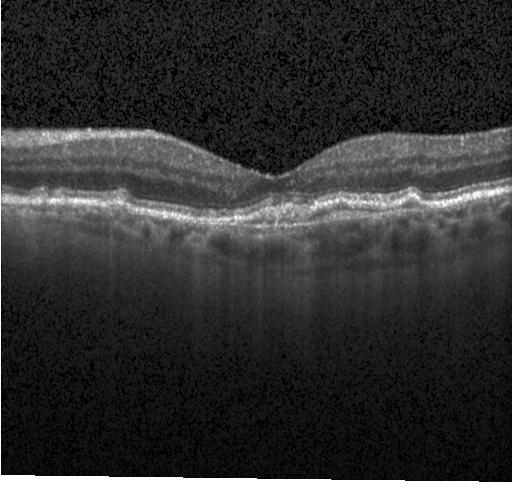

Retinal OCT cross-section · horizontal scan through the fovea
Impression: a choroidal neovascular membrane.